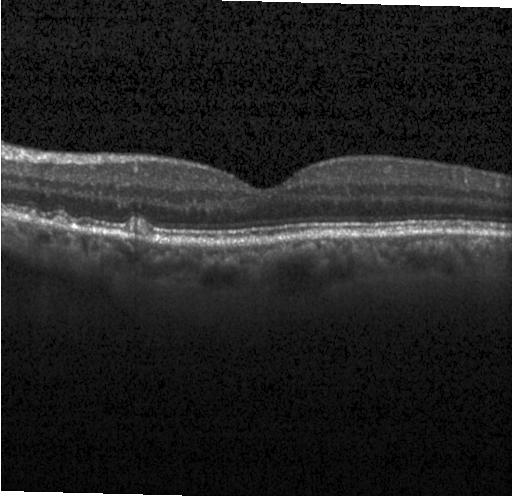

Finding: multiple drusen.